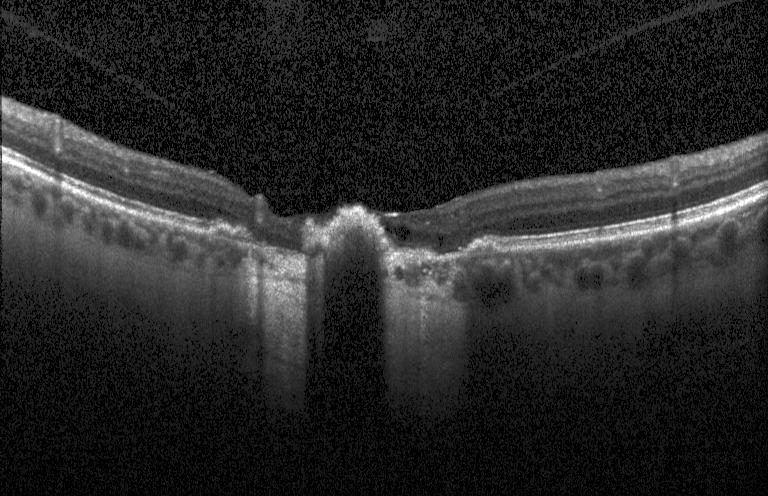 Retinal OCT B-scan; Heidelberg Spectralis; horizontal scan through the fovea — Finding: a choroidal neovascular membrane.